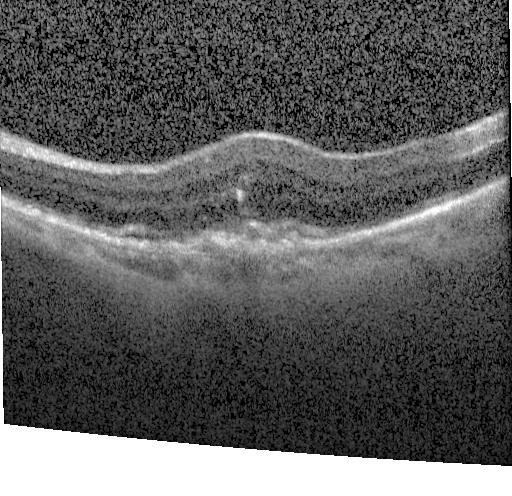 Diagnosis: a choroidal neovascular membrane.